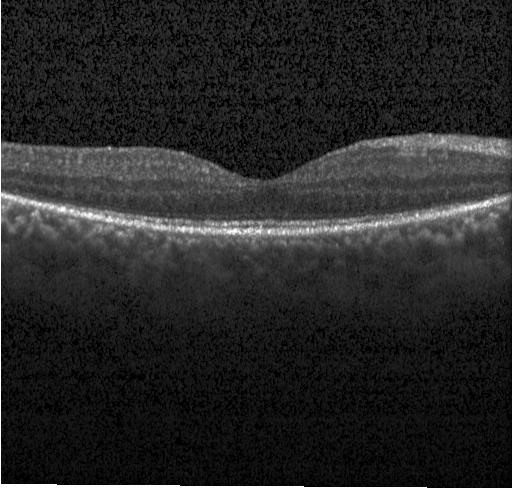

Spectral-domain optical coherence tomography · through the macula · Heidelberg Spectralis OCT system · retinal OCT cross-section. Assessment: neither choroidal neovascularization, diabetic macular edema, nor drusen.